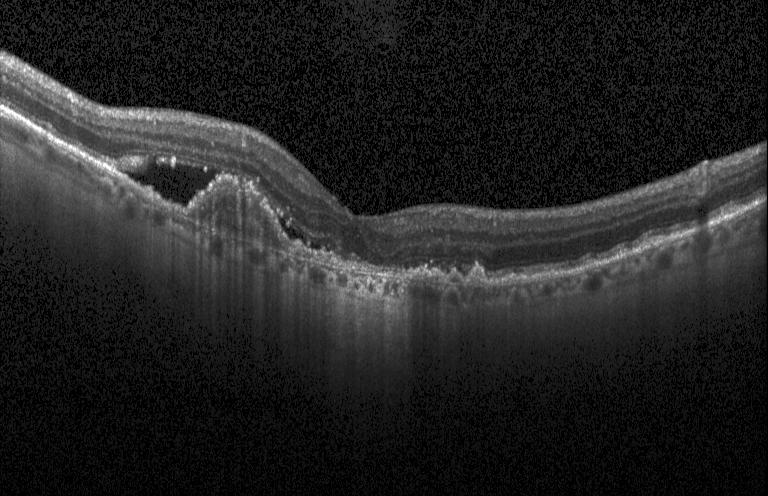 Optical coherence tomography scan.
Macular OCT: choroidal neovascularization.